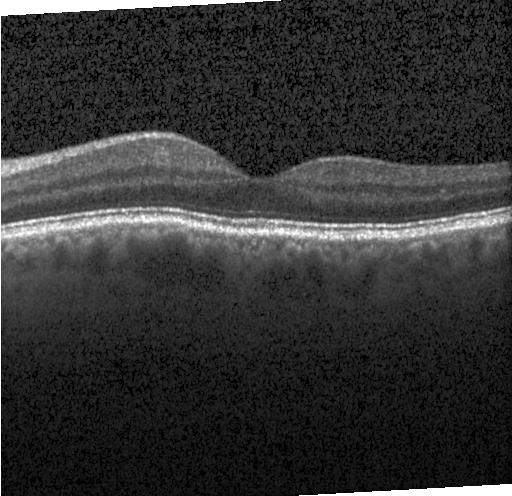
Macular OCT: no choroidal neovascularization, diabetic macular edema, or drusen.